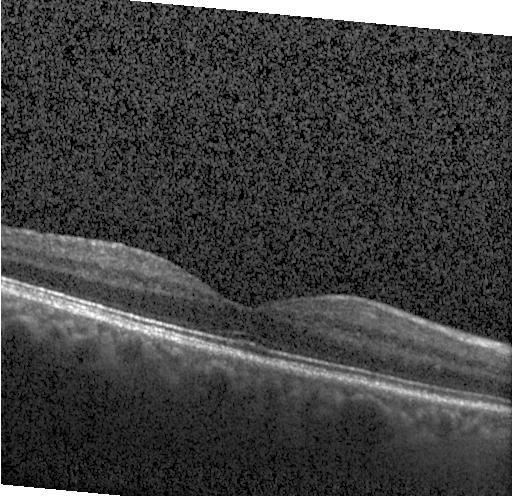

Macular scan; spectral-domain optical coherence tomography; instrument: Heidelberg Spectralis; retinal OCT cross-section.
The scan shows no choroidal neovascularization, no diabetic macular edema, and no drusen.